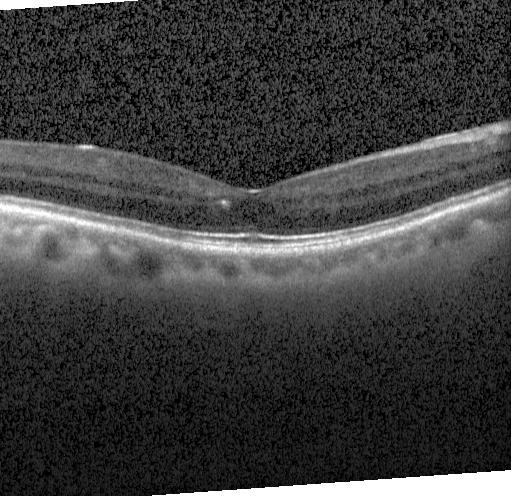
Assessment: no CNV, DME, or drusen.